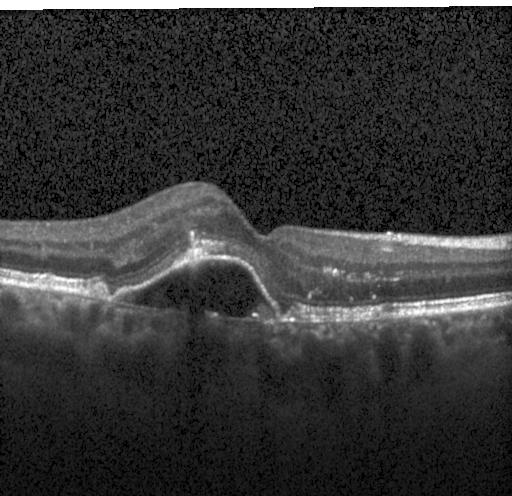

Finding: CNV.